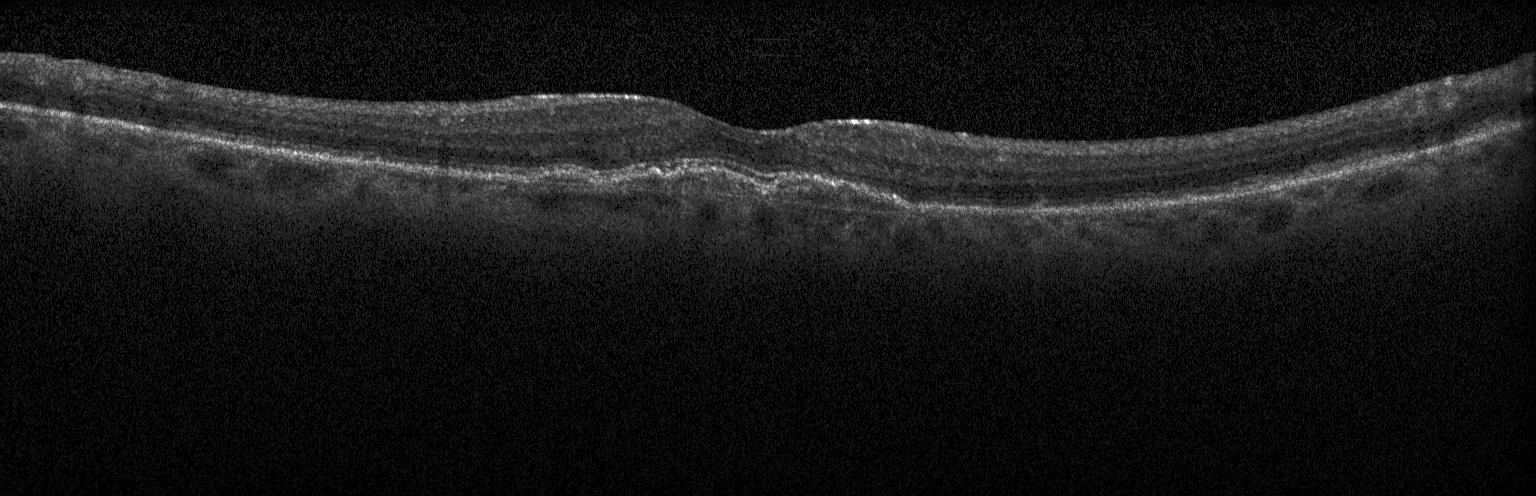
Spectral-domain OCT · through the macula · retinal OCT B-scan · instrument: Heidelberg Spectralis.
Diagnosis: a choroidal neovascular membrane.